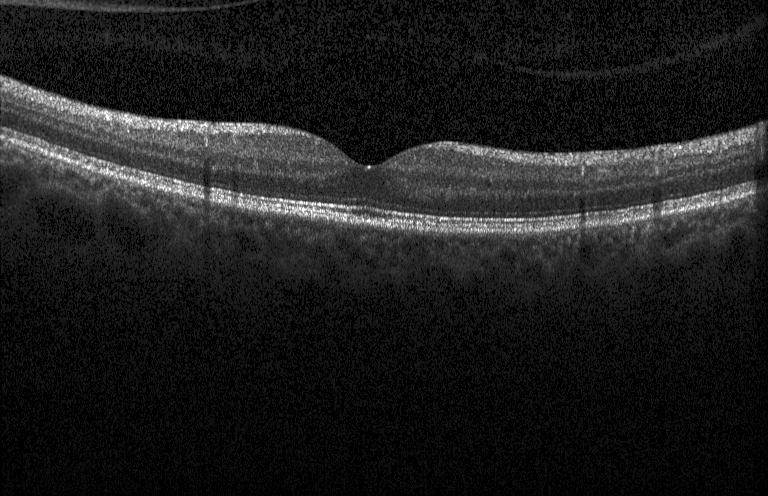

Retinal OCT cross-section showing no choroidal neovascularization, diabetic macular edema, or drusen.